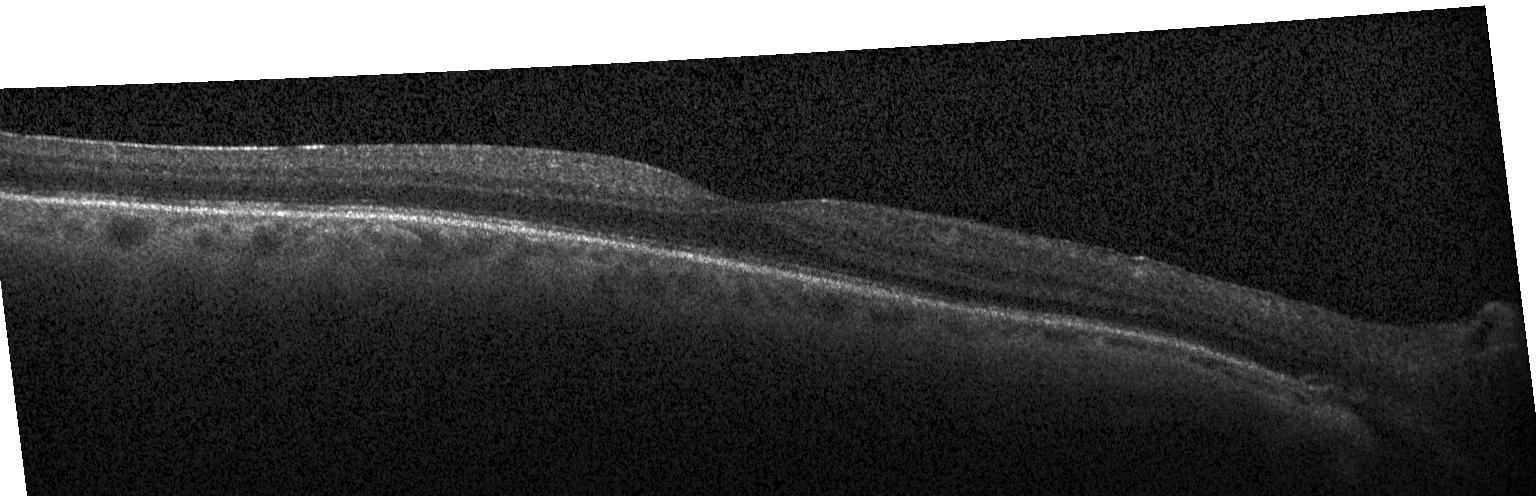

Optical coherence tomography scan · spectral-domain optical coherence tomography
The scan shows neither choroidal neovascularization, diabetic macular edema, nor drusen.